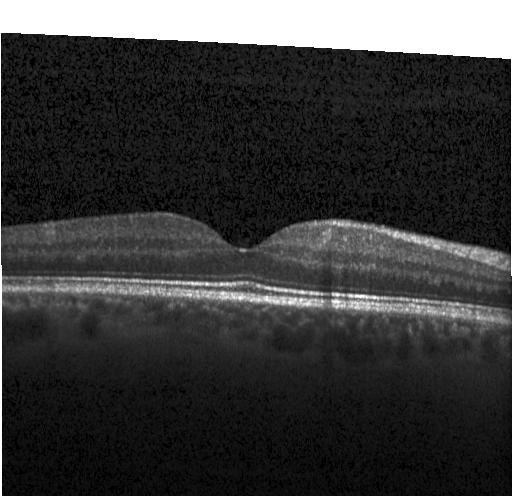

Finding: neither CNV, DME, nor drusen.